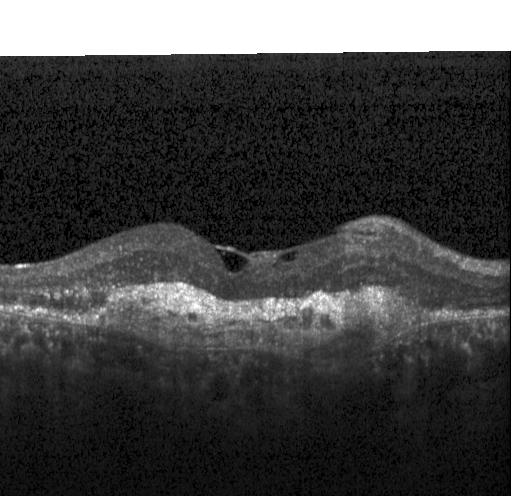
Optical coherence tomography B-scan; spectral-domain OCT.
Finding: choroidal neovascularization (CNV).